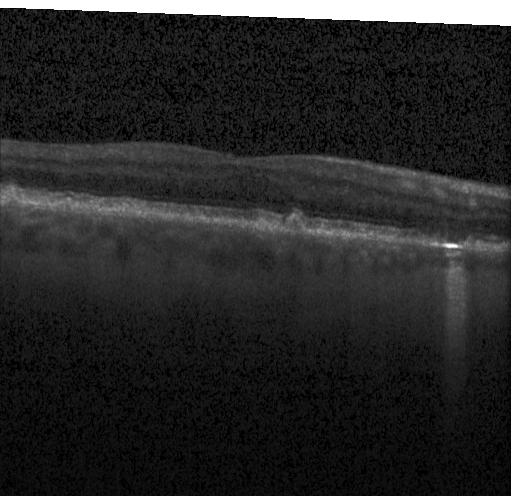
Impression: sub-RPE drusenoid deposits.